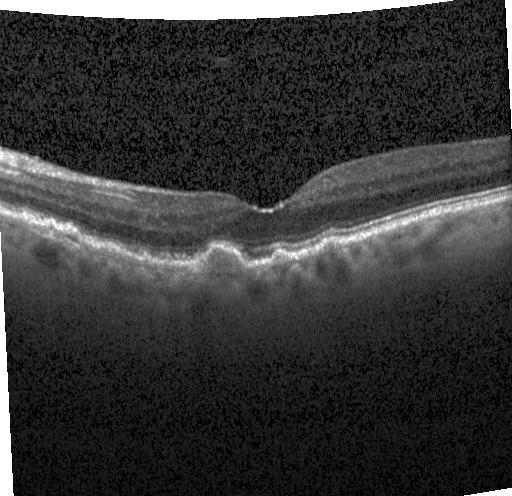

Macular scan, optical coherence tomography scan — Dx: multiple drusen.